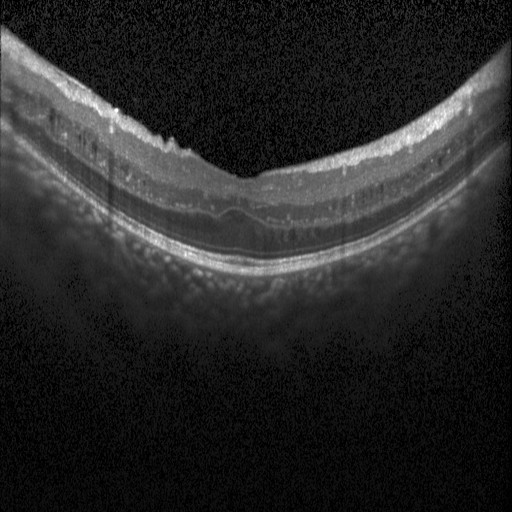

OCT finding: diabetic macular edema (DME).